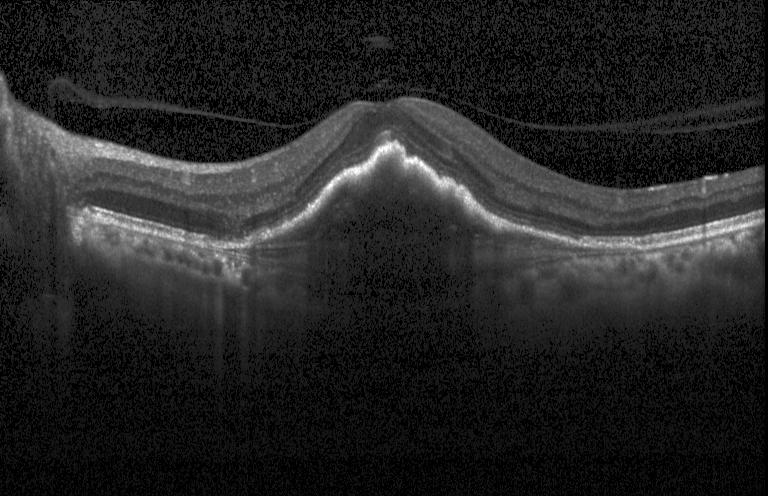

Macular OCT demonstrating choroidal neovascularization.